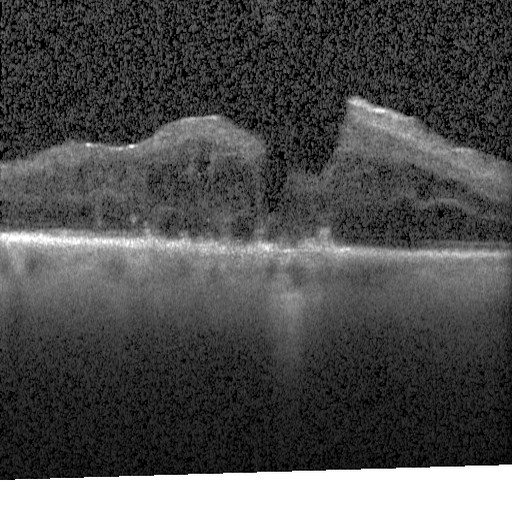
Spectral-domain OCT. Optical coherence tomography B-scan — Impression: diabetic macular edema (DME).